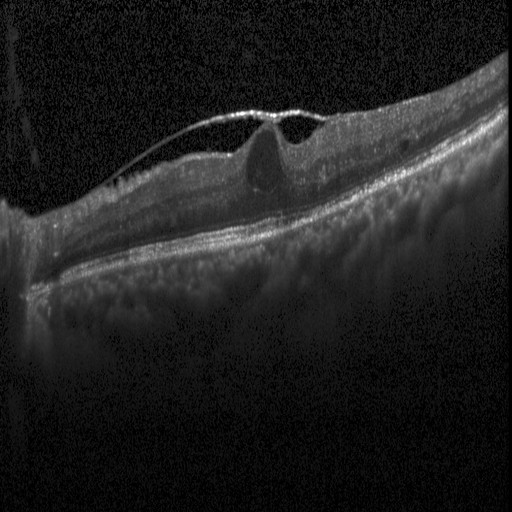
Optical coherence tomography scan — The scan shows diabetic macular edema (DME).